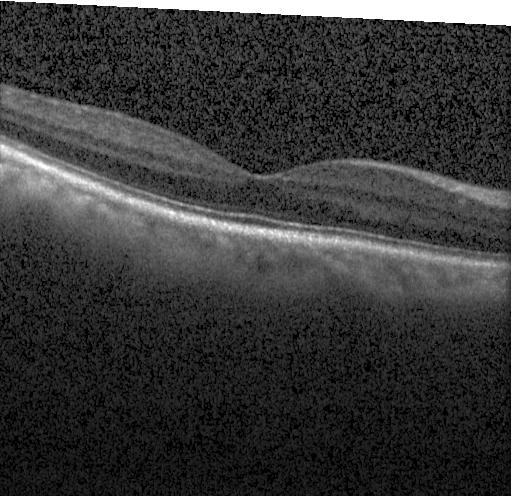
Spectral-domain optical coherence tomography · Heidelberg Spectralis · retinal OCT cross-section. This B-scan demonstrates no evidence of choroidal neovascularization, diabetic macular edema, or drusen.